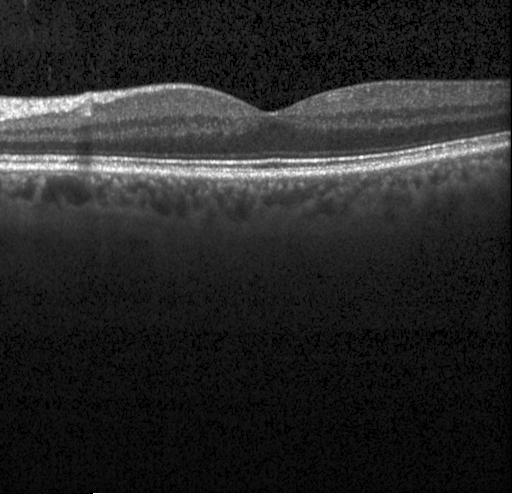

Fovea-centered; spectral-domain OCT; retinal OCT cross-section; Heidelberg Spectralis
Impression: no choroidal neovascularization, diabetic macular edema, or drusen.